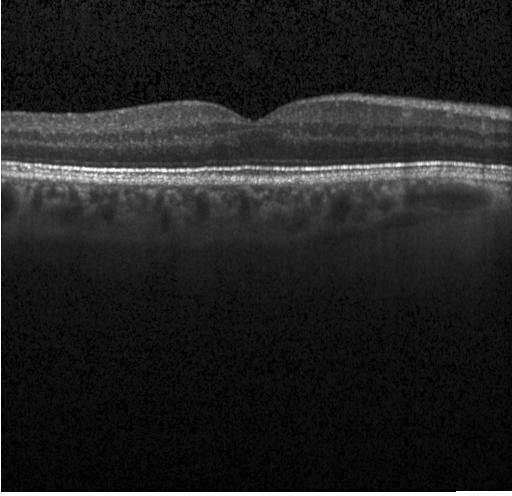

Through the macula · OCT line scan · SD-OCT · Heidelberg Spectralis.
Finding: no evidence of CNV, DME, or drusen.